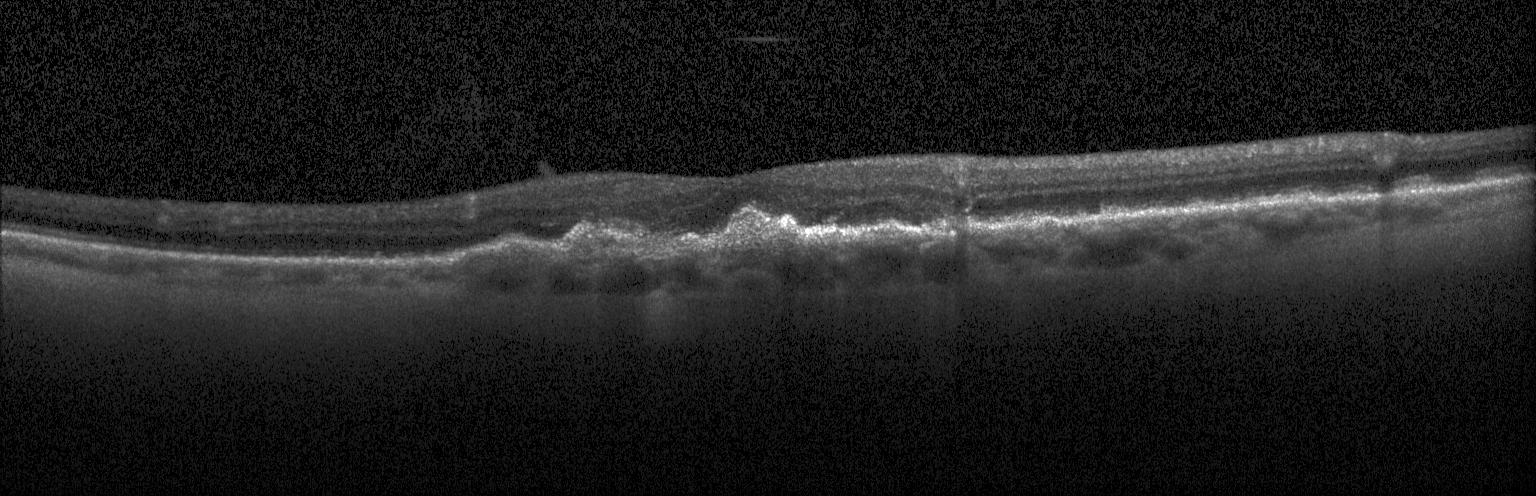
Dx: choroidal neovascularization.